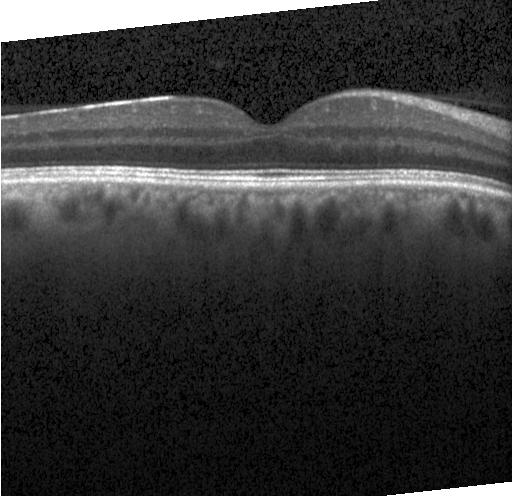

Impression: no evidence of CNV, DME, or drusen.